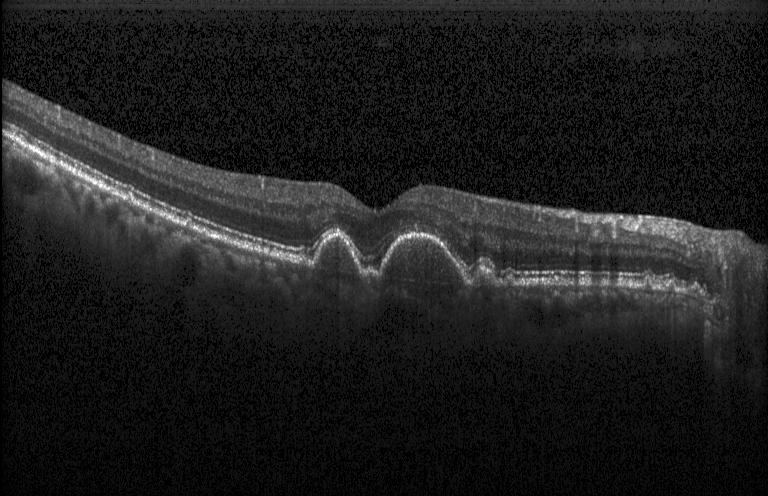

OCT scan showing drusen.